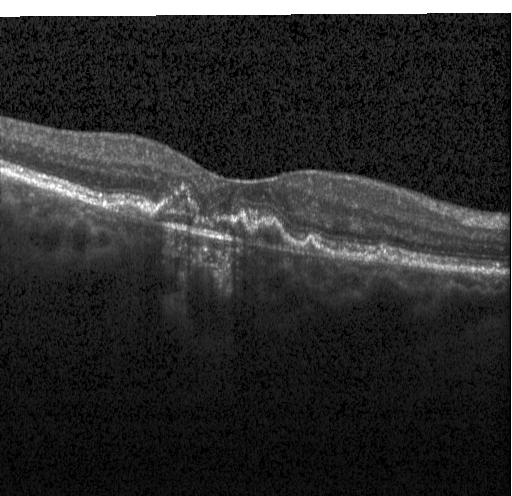
Horizontal scan through the fovea; OCT line scan; Heidelberg Spectralis OCT system; SD-OCT.
Dx: choroidal neovascularization (CNV).